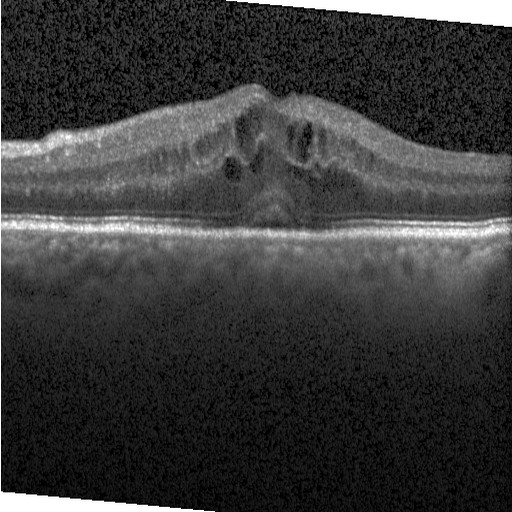

Impression: diabetic macular edema.